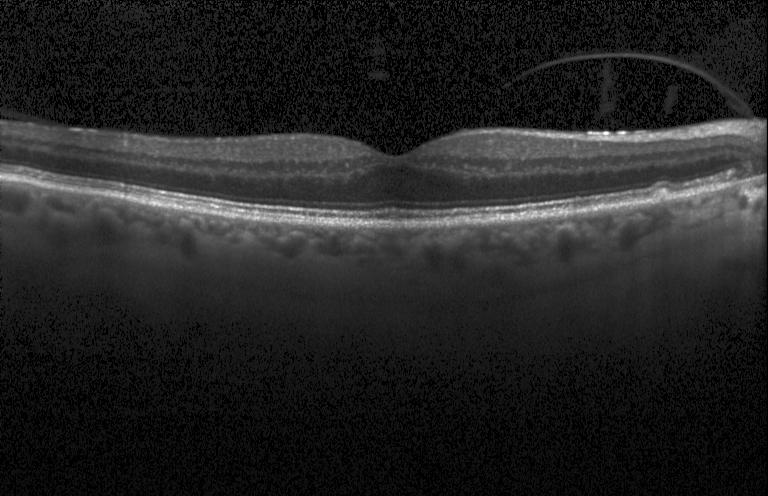 OCT finding: no evidence of CNV, DME, or drusen.